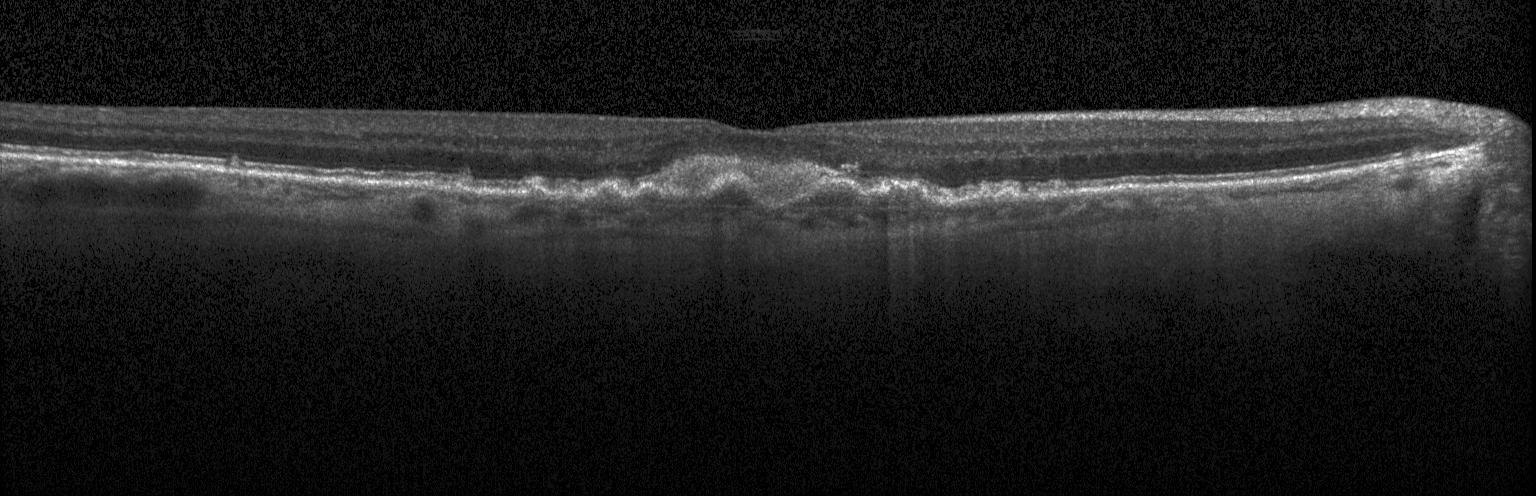 Centered on the fovea; optical coherence tomography scan — This B-scan demonstrates choroidal neovascularization.